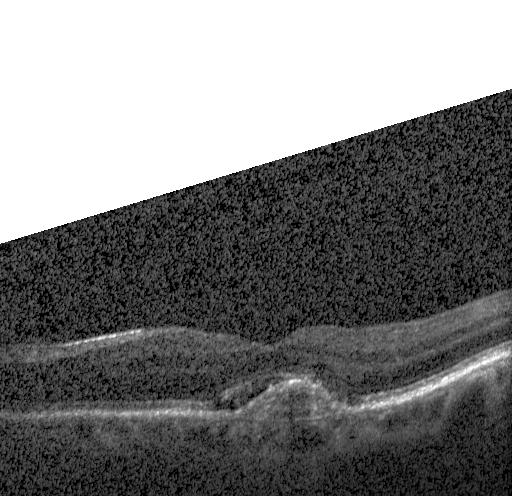 OCT B-scan · acquired on a Heidelberg Spectralis · fovea-centered.
Impression: a choroidal neovascular membrane.